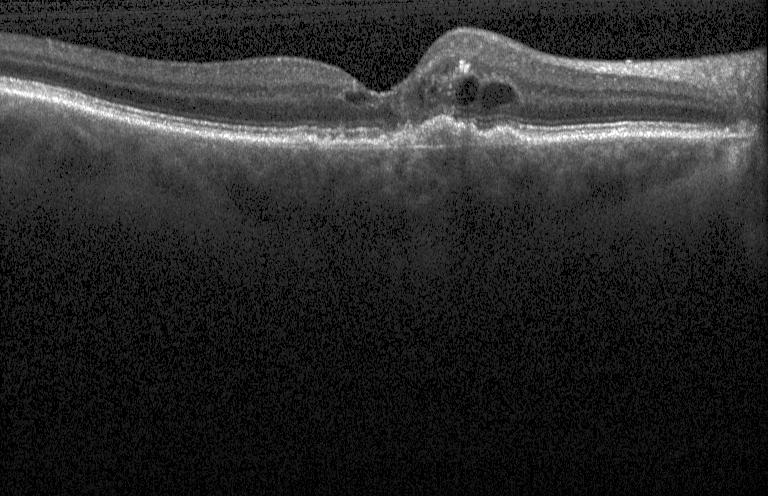
Impression: choroidal neovascularization.